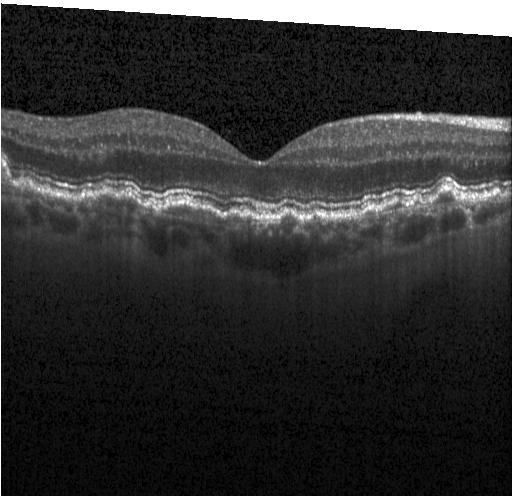
Retinal OCT cross-section. OCT finding: sub-RPE drusenoid deposits.